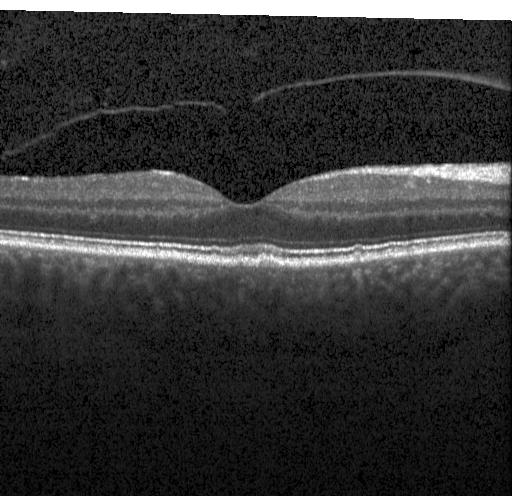
Heidelberg Spectralis, optical coherence tomography B-scan.
Diagnosis: sub-RPE drusenoid deposits.